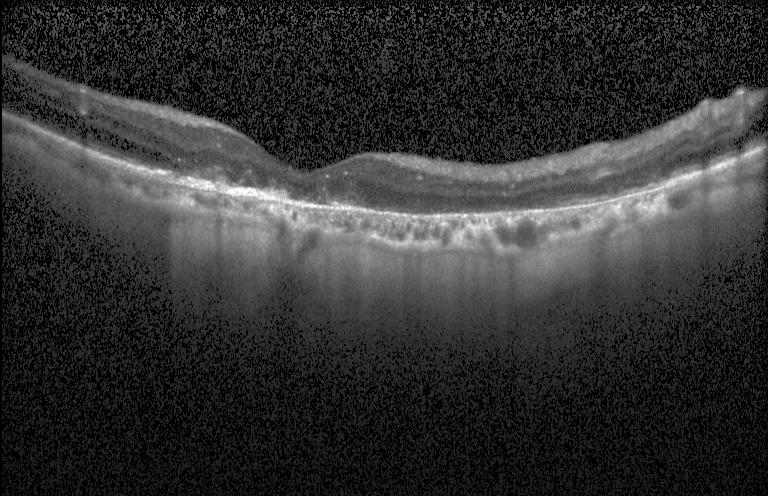
Assessment: CNV.